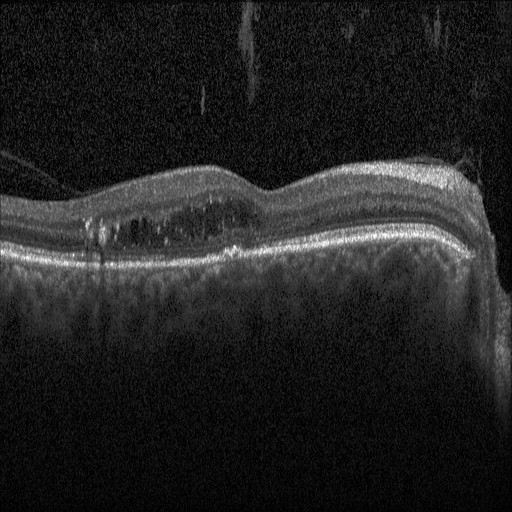 Spectral-domain OCT B-scan: DME.